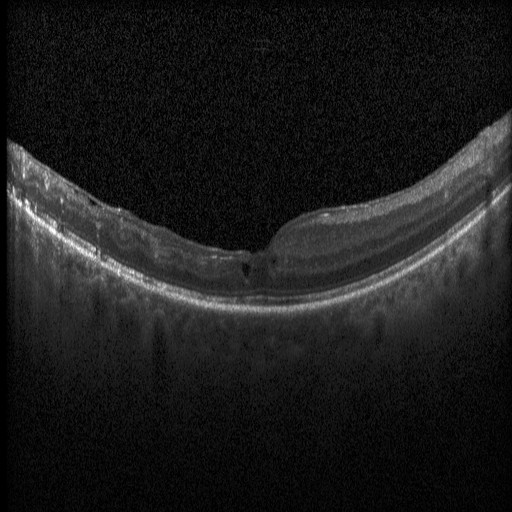
Retinal OCT B-scan — Impression: diabetic macular edema.